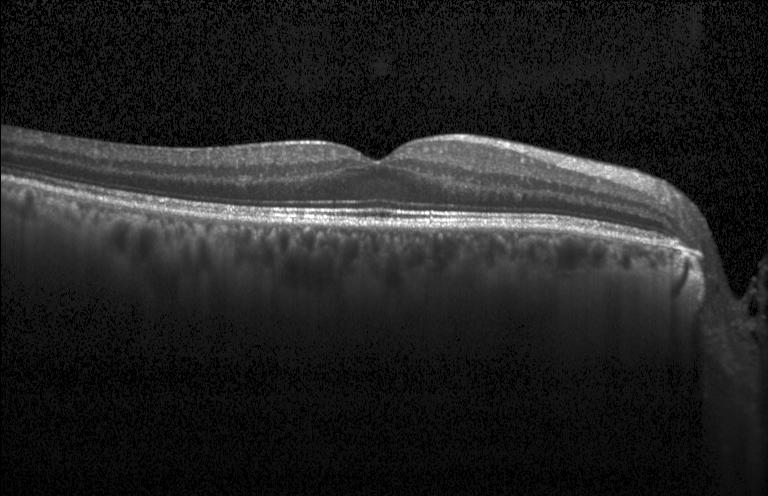

Instrument: Heidelberg Spectralis · optical coherence tomography scan.
The scan shows no choroidal neovascularization, diabetic macular edema, or drusen.